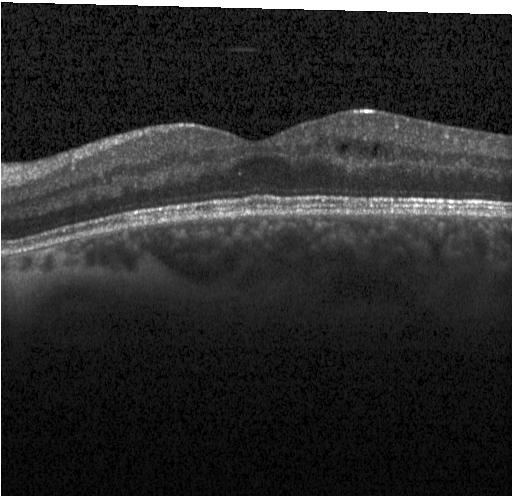 SD-OCT; through the macula; OCT B-scan. Macular OCT: diabetic macular edema.